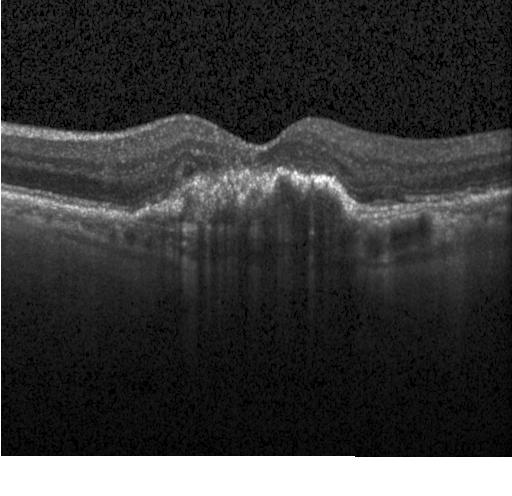 Finding: choroidal neovascularization.